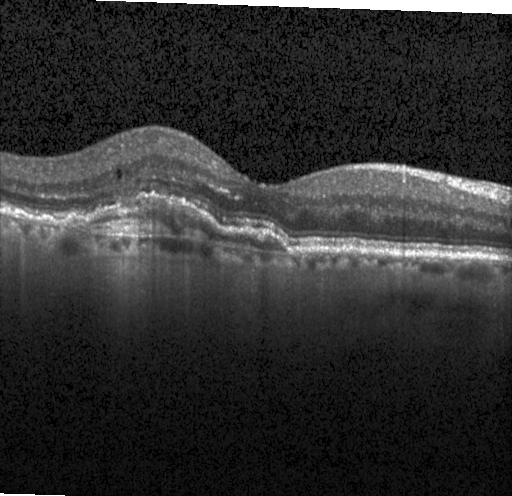 Macular OCT: a choroidal neovascular membrane.